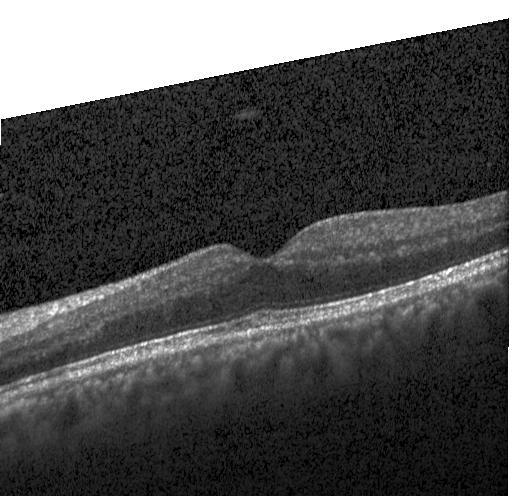
OCT B-scan showing no evidence of choroidal neovascularization, diabetic macular edema, or drusen.